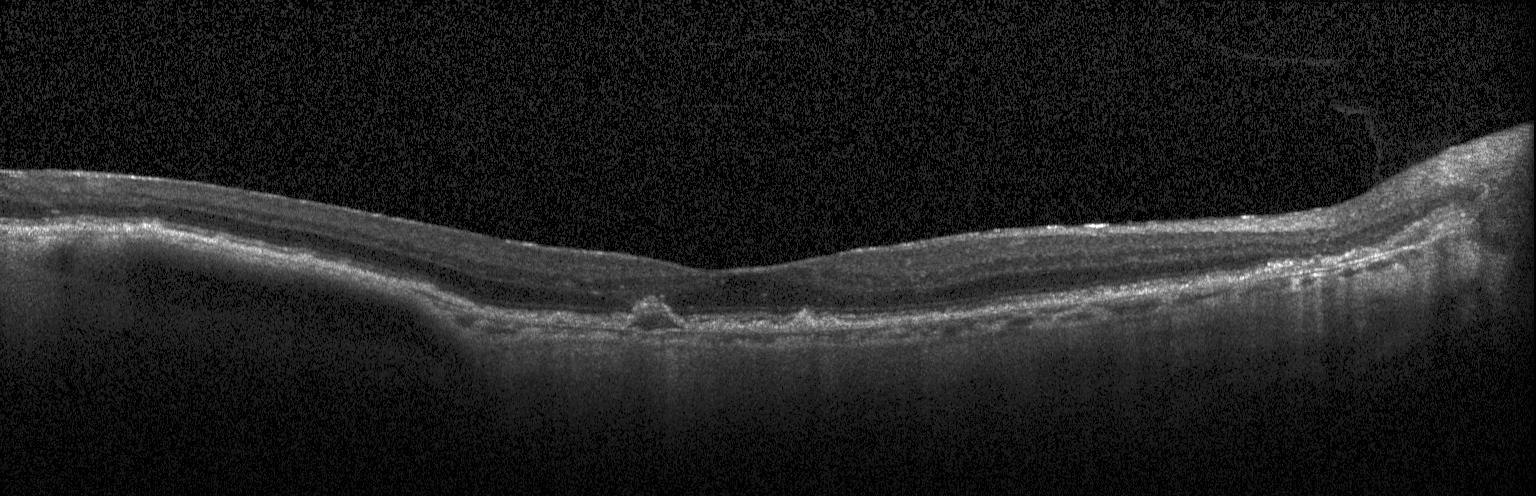 OCT B-scan; spectral-domain optical coherence tomography; acquired on a Heidelberg Spectralis; macular scan
A choroidal neovascular membrane.